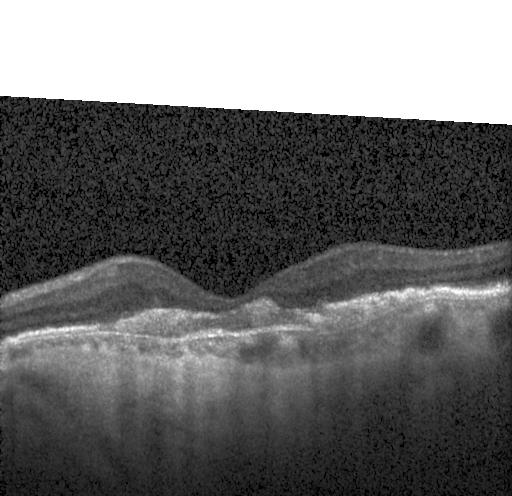 Diagnosis: a choroidal neovascular membrane.